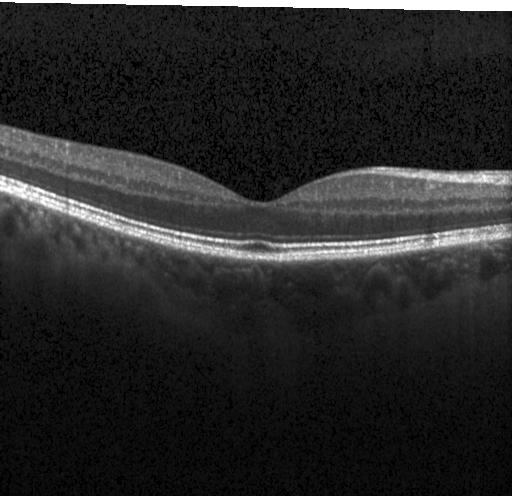
Macular OCT demonstrating no choroidal neovascularization, diabetic macular edema, or drusen.